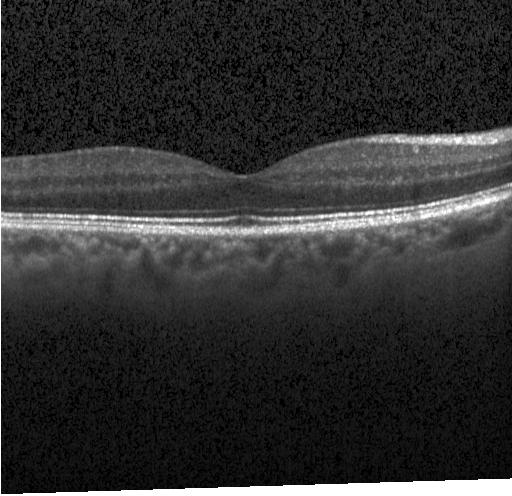
OCT line scan. Diagnosis: no evidence of CNV, DME, or drusen.